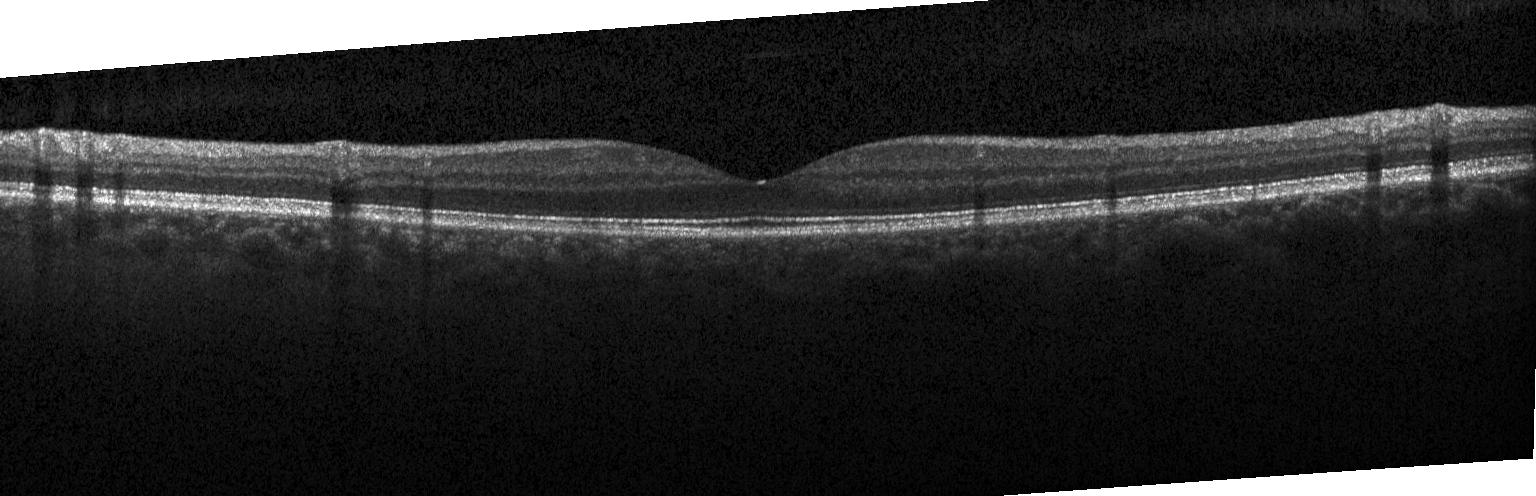
Macular OCT demonstrating neither choroidal neovascularization, diabetic macular edema, nor drusen.